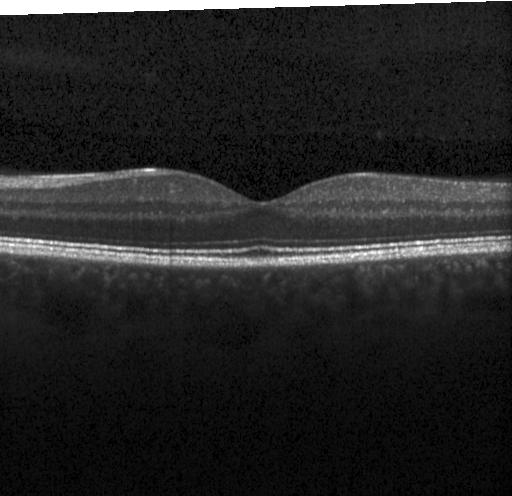

Impression: no choroidal neovascularization, diabetic macular edema, or drusen.